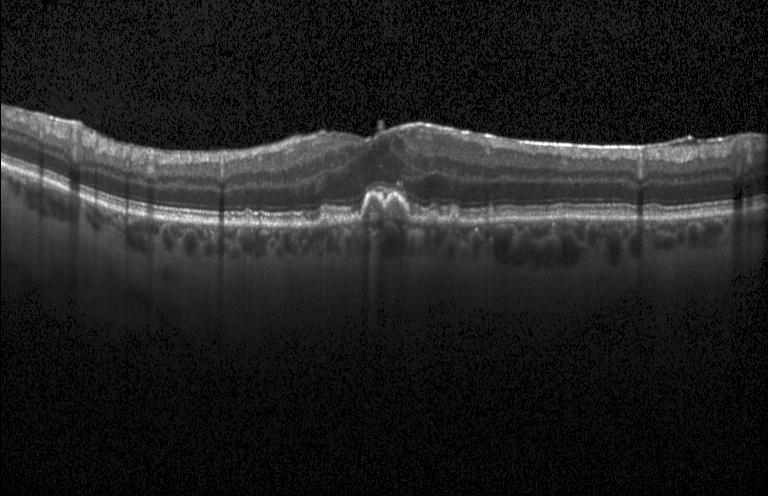
Macular OCT: multiple drusen.